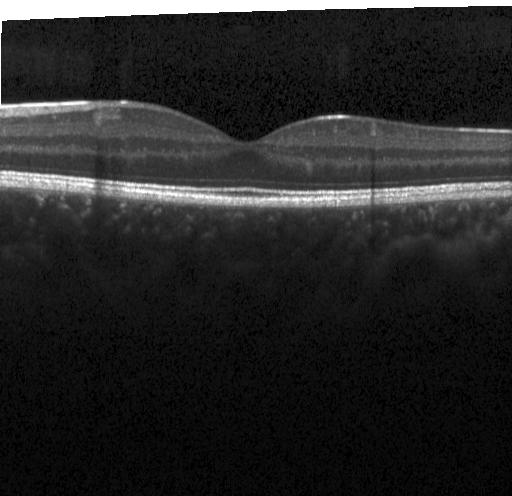

Optical coherence tomography scan; horizontal scan through the fovea; Heidelberg Spectralis.
Finding: no CNV, DME, or drusen.